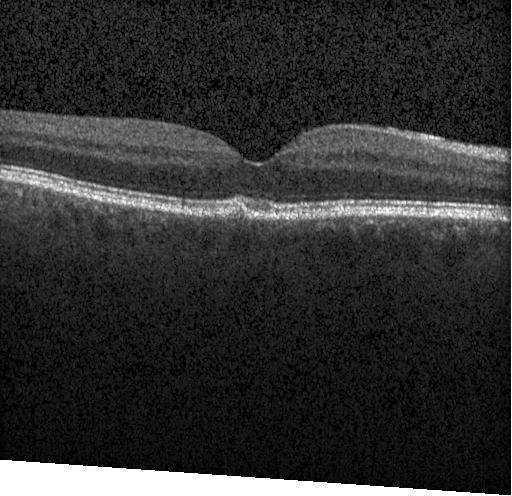
Diagnosis: multiple drusen.